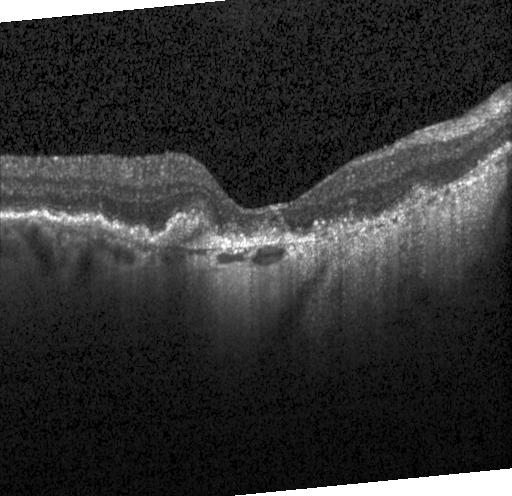
Heidelberg Spectralis OCT system, SD-OCT, horizontal scan through the fovea, OCT B-scan
Impression: choroidal neovascularization.